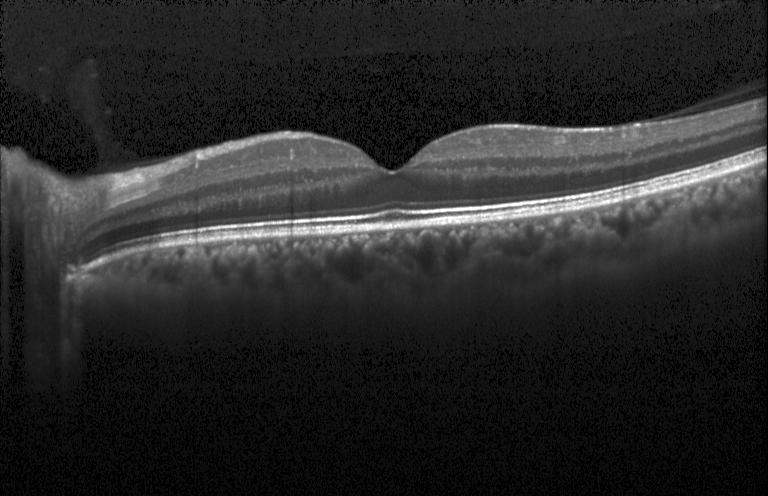

Instrument: Heidelberg Spectralis, horizontal scan through the fovea, retinal OCT cross-section, spectral-domain OCT. Diagnosis: neither choroidal neovascularization, diabetic macular edema, nor drusen.